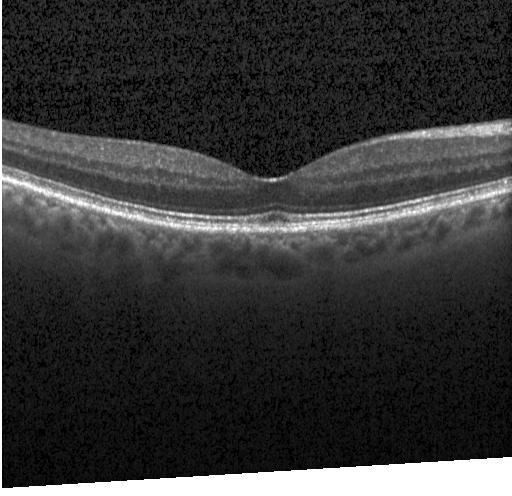 Retinal OCT cross-section showing no choroidal neovascularization, no diabetic macular edema, and no drusen.